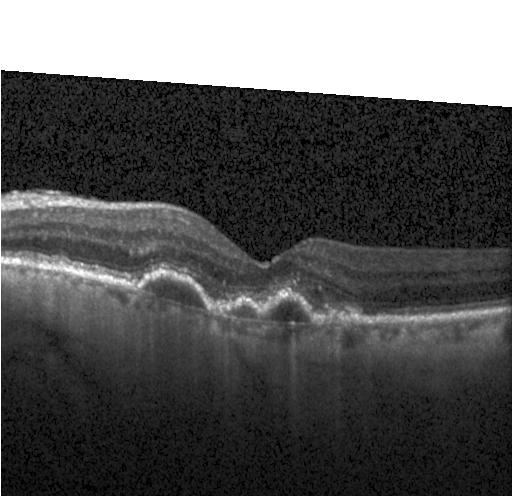 Retinal OCT B-scan. Impression: a choroidal neovascular membrane.